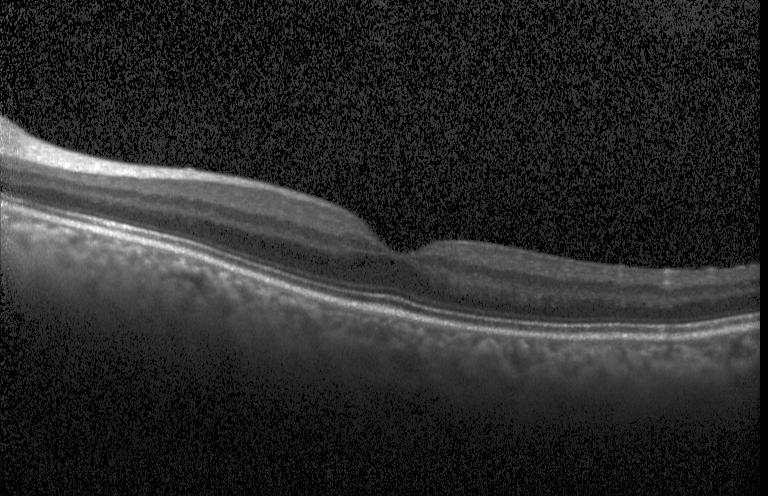
OCT scan showing no CNV, DME, or drusen.